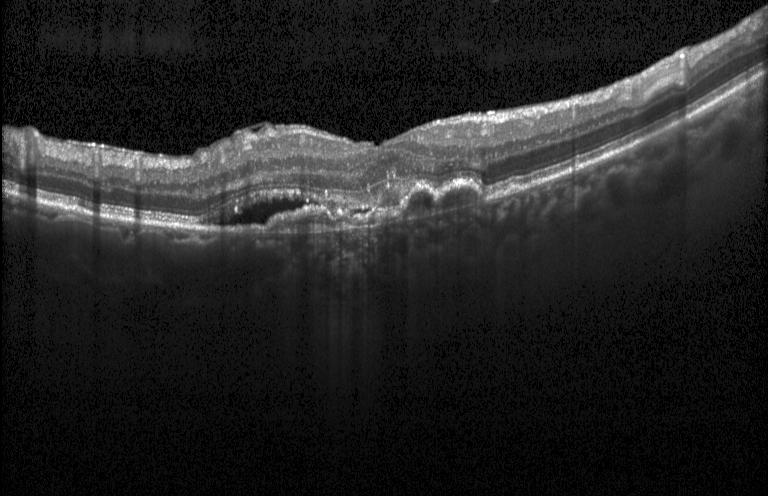
OCT line scan, horizontal scan through the fovea — Assessment: a choroidal neovascular membrane.